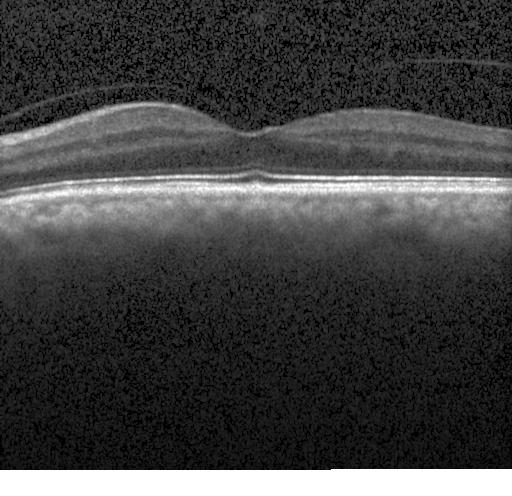

SD-OCT · Heidelberg Spectralis OCT system · centered on the fovea · optical coherence tomography B-scan — Dx: neither CNV, DME, nor drusen.